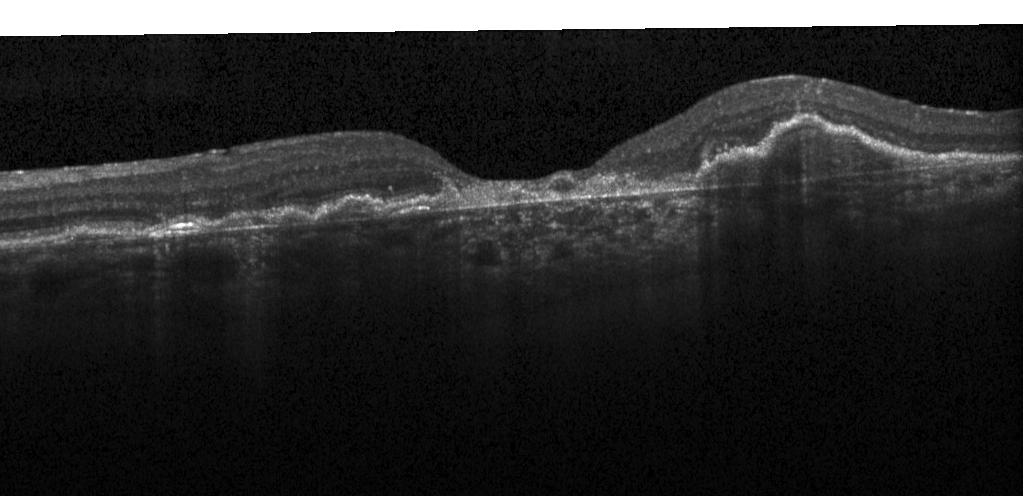
Heidelberg Spectralis; spectral-domain optical coherence tomography; OCT line scan
Impression: CNV.